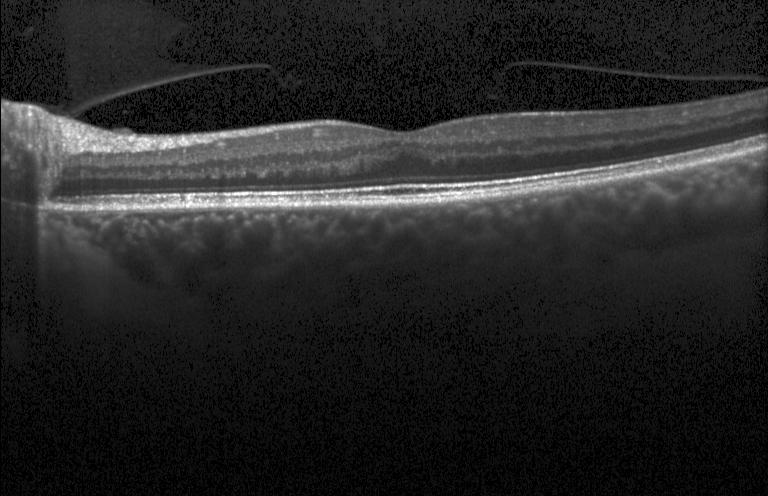 Instrument: Heidelberg Spectralis · retinal OCT cross-section
No choroidal neovascularization, diabetic macular edema, or drusen.